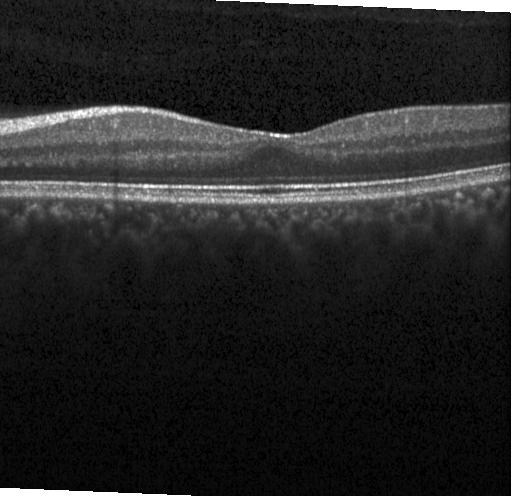 Impression: neither choroidal neovascularization, diabetic macular edema, nor drusen.